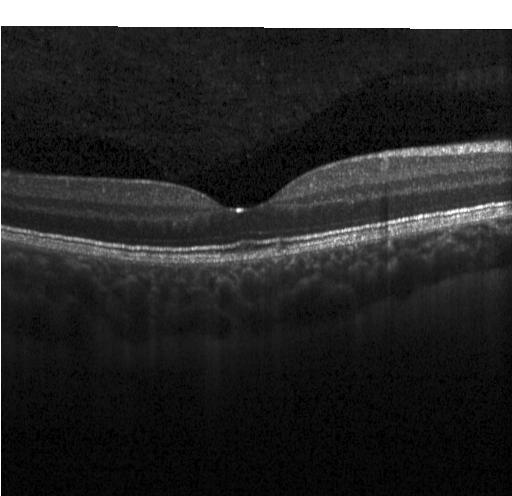

OCT B-scan
Assessment: no choroidal neovascularization, no diabetic macular edema, and no drusen.